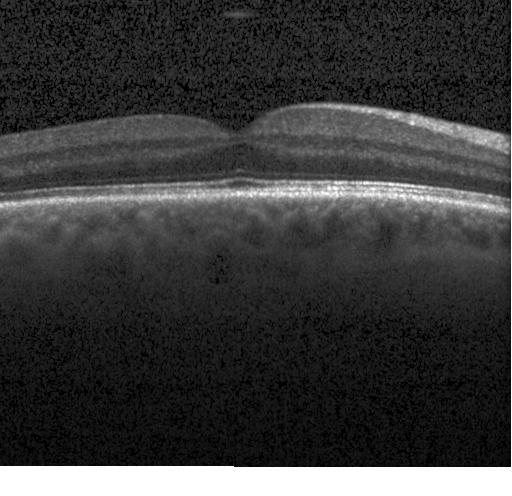

Centered on the fovea. Optical coherence tomography scan — The scan shows neither choroidal neovascularization, diabetic macular edema, nor drusen.